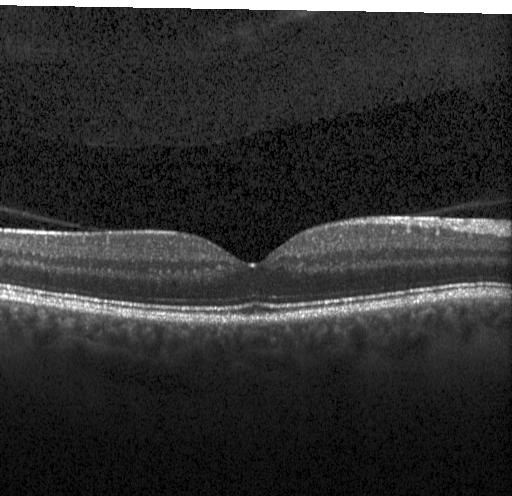
Acquired on a Heidelberg Spectralis; retinal OCT cross-section. Assessment: no choroidal neovascularization, diabetic macular edema, or drusen.